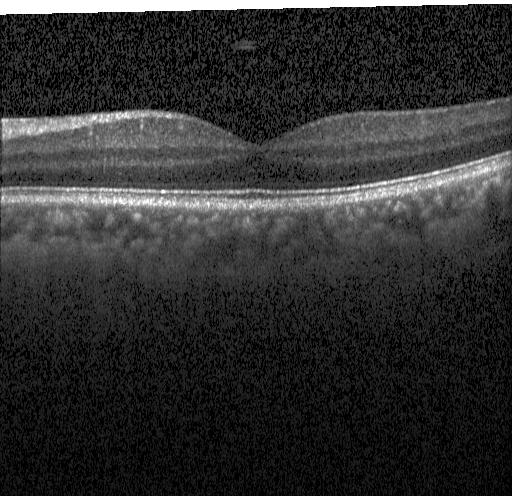 Fovea-centered; acquired on a Heidelberg Spectralis; retinal OCT cross-section.
Diagnosis: no CNV, DME, or drusen.